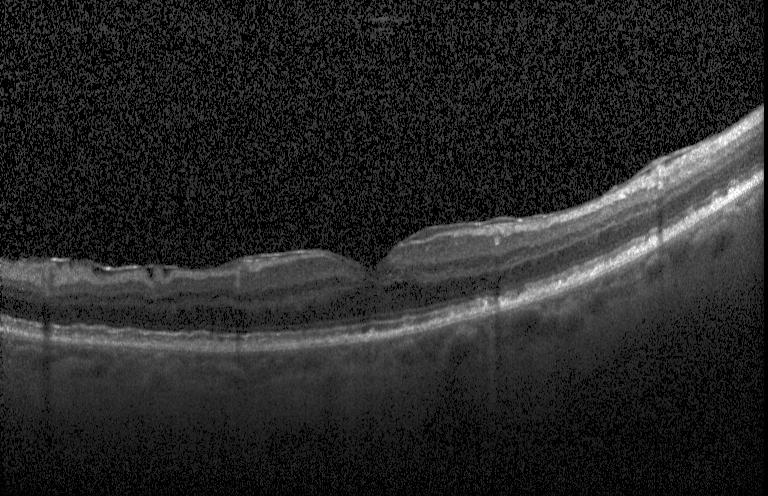

Spectral-domain OCT. OCT line scan. Through the macula
Impression: multiple drusen.